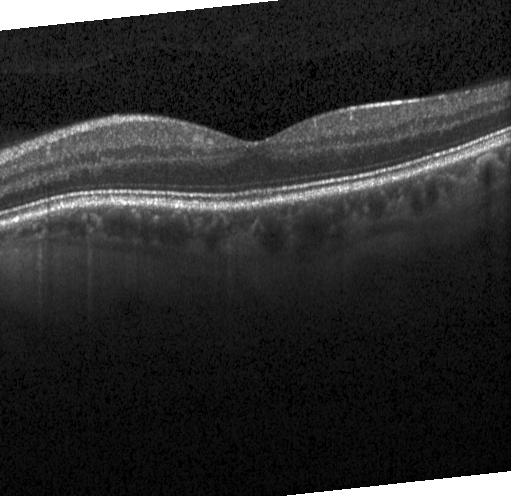

Retinal OCT cross-section showing no CNV, DME, or drusen.